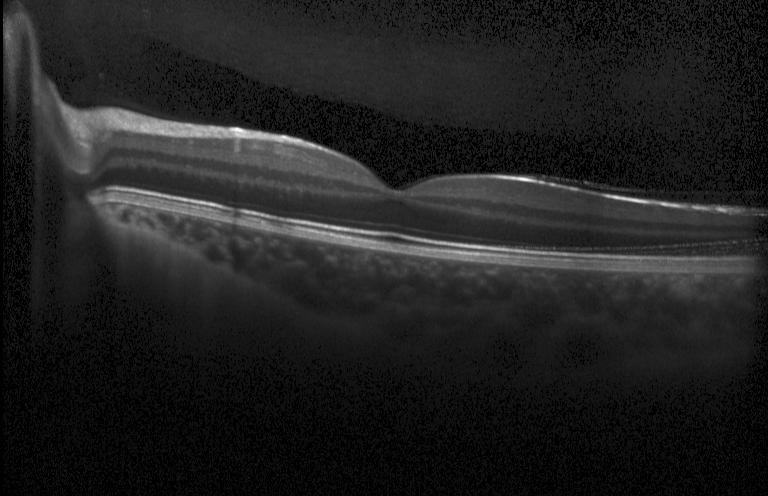 Spectral-domain OCT B-scan: neither CNV, DME, nor drusen.